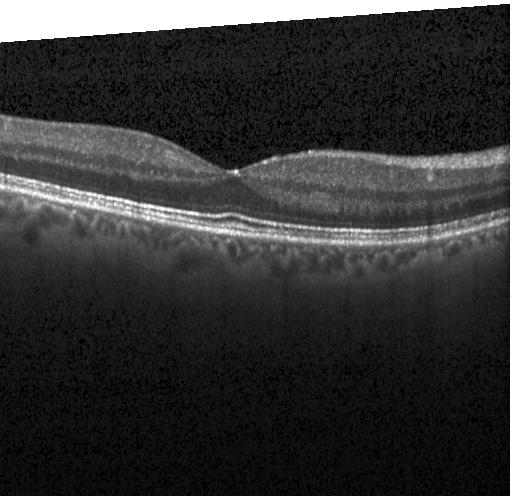 OCT finding: no evidence of choroidal neovascularization, diabetic macular edema, or drusen.